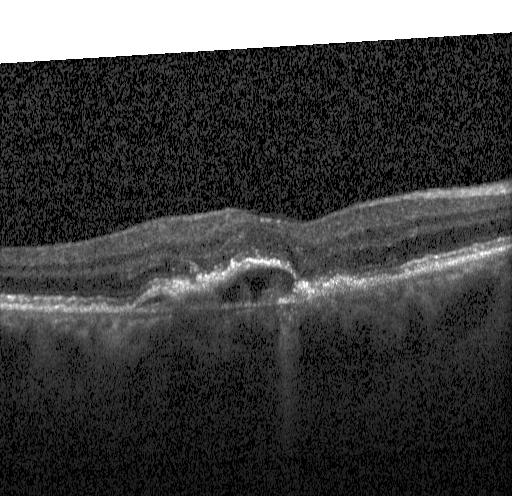

Spectral-domain optical coherence tomography. Heidelberg Spectralis OCT system. Through the macula. OCT B-scan.
This B-scan demonstrates a choroidal neovascular membrane.